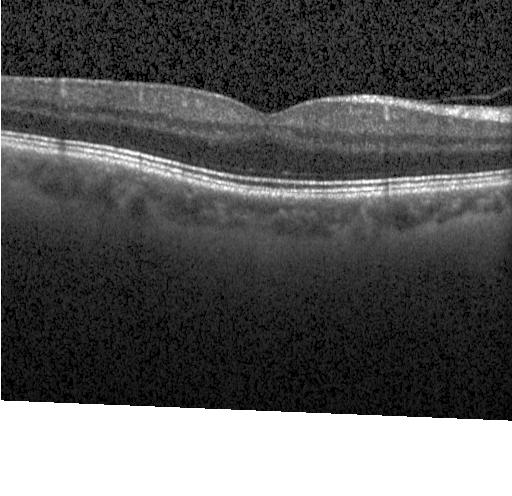
OCT line scan · SD-OCT · acquired on a Heidelberg Spectralis.
No evidence of CNV, DME, or drusen.